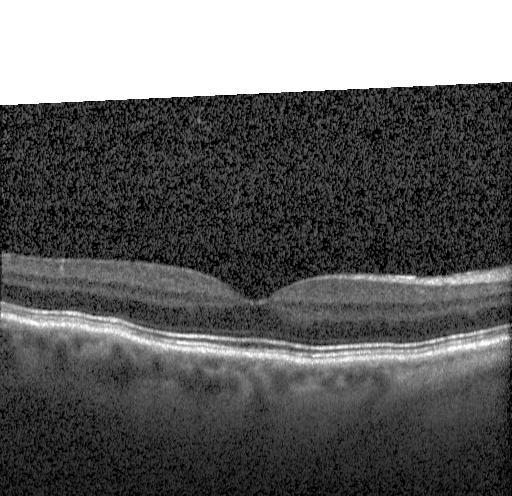
OCT scan showing no CNV, no DME, and no drusen.